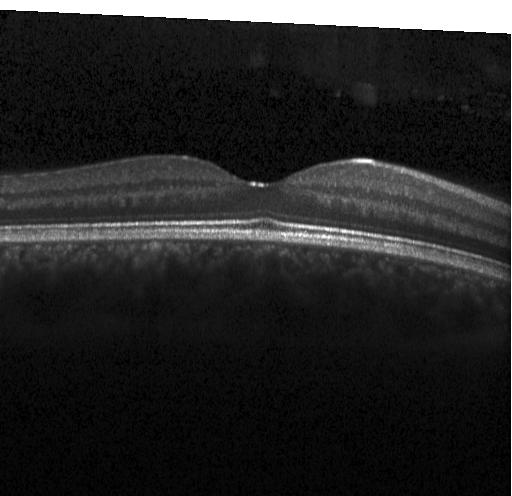 Spectral-domain OCT B-scan: no choroidal neovascularization, no diabetic macular edema, and no drusen.